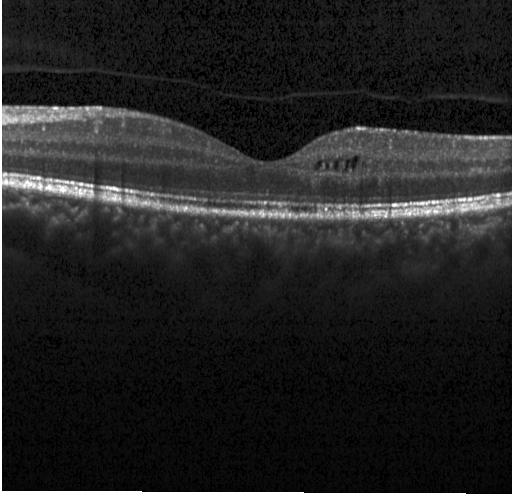 Retinal OCT cross-section. Diagnosis: diabetic macular edema (DME).